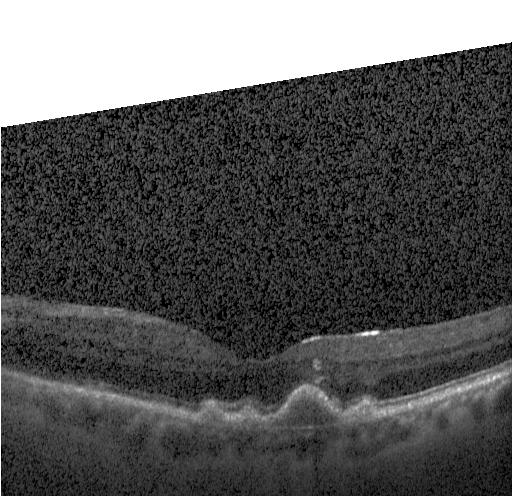 Acquired on a Heidelberg Spectralis; OCT B-scan. Assessment: sub-RPE drusenoid deposits.